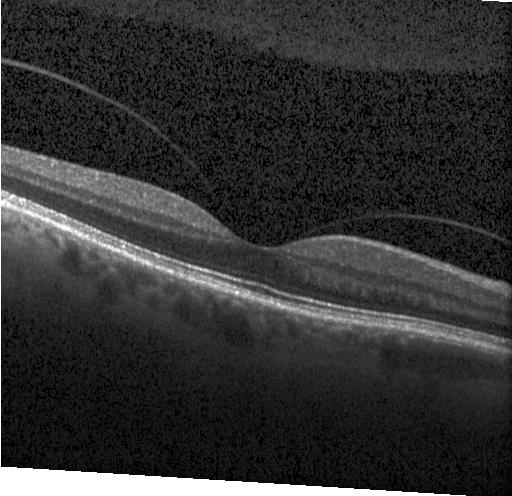

Heidelberg Spectralis OCT system. Horizontal scan through the fovea. Retinal OCT B-scan — Assessment: no choroidal neovascularization, diabetic macular edema, or drusen.